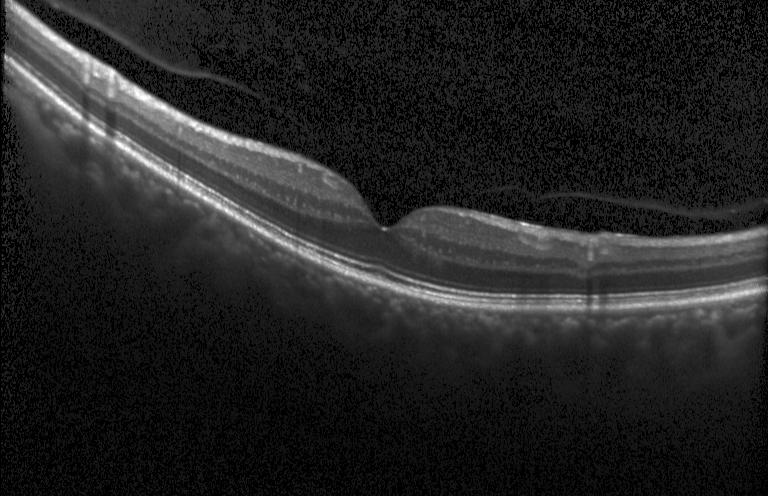 Retinal OCT cross-section. Spectral-domain optical coherence tomography. Through the macula.
Macular OCT: neither CNV, DME, nor drusen.